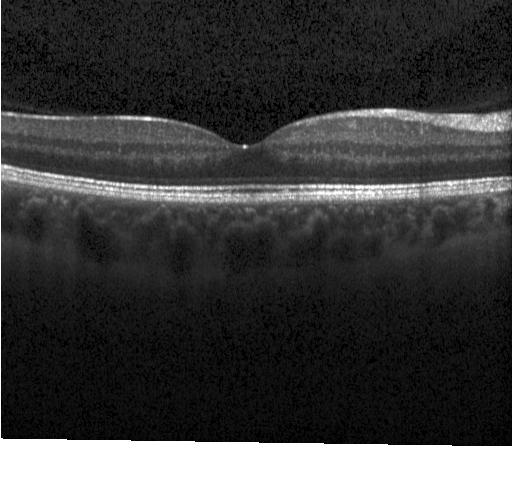

Retinal OCT B-scan · centered on the fovea
Dx: neither choroidal neovascularization, diabetic macular edema, nor drusen.